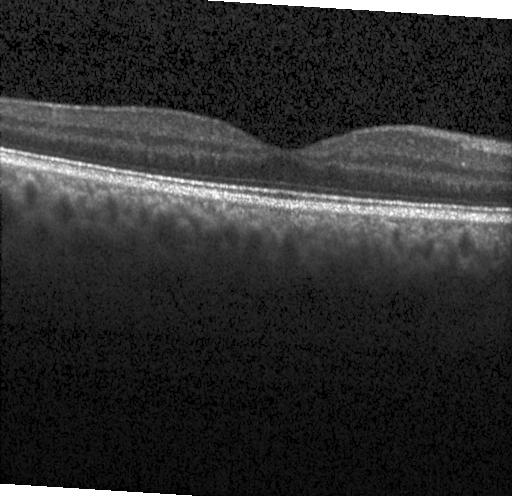
Diagnosis: no choroidal neovascularization, diabetic macular edema, or drusen.